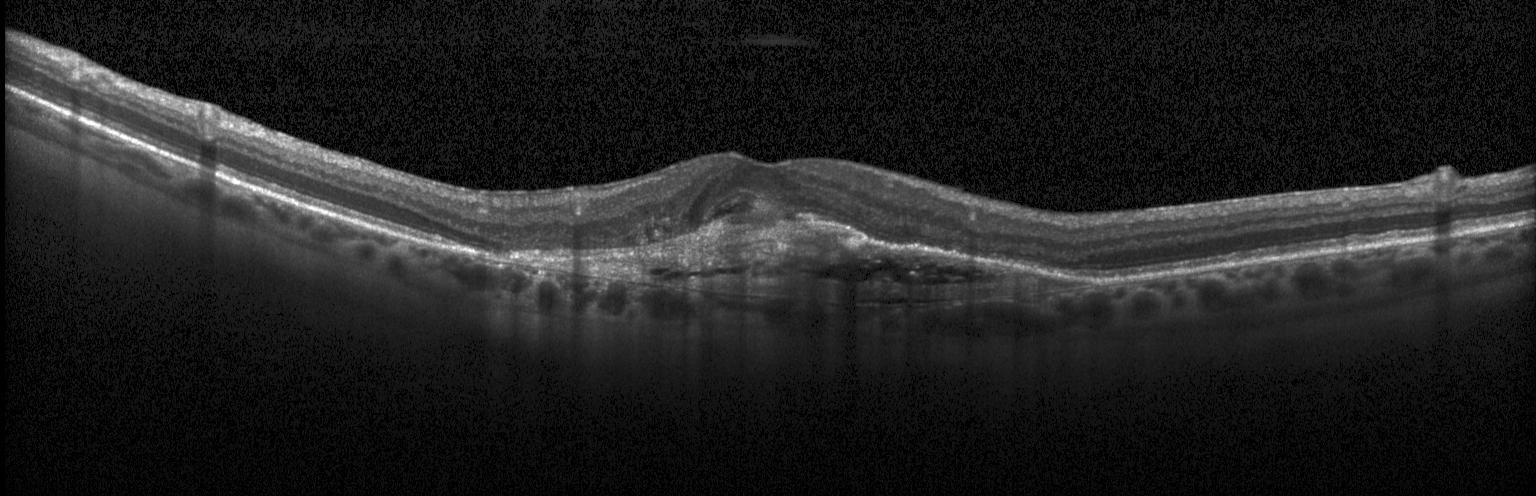

Heidelberg Spectralis OCT system. Optical coherence tomography B-scan
OCT finding: choroidal neovascularization (CNV).